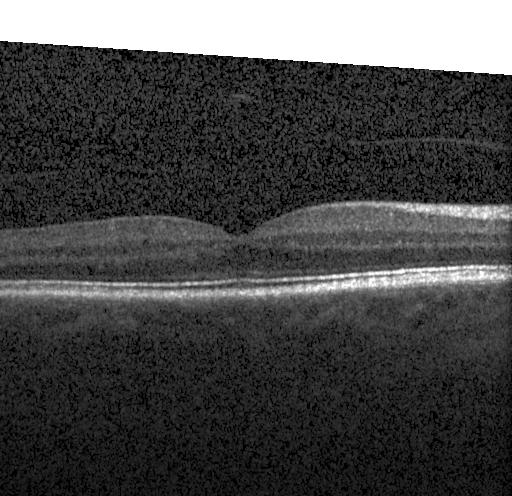
Spectral-domain OCT. OCT line scan. Macular scan. Heidelberg Spectralis OCT system. Finding: no evidence of CNV, DME, or drusen.